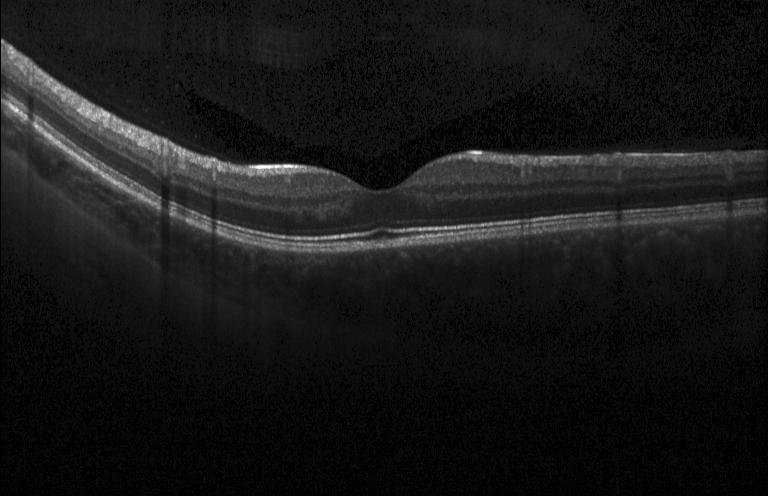

Spectral-domain OCT. OCT B-scan. Assessment: no evidence of CNV, DME, or drusen.